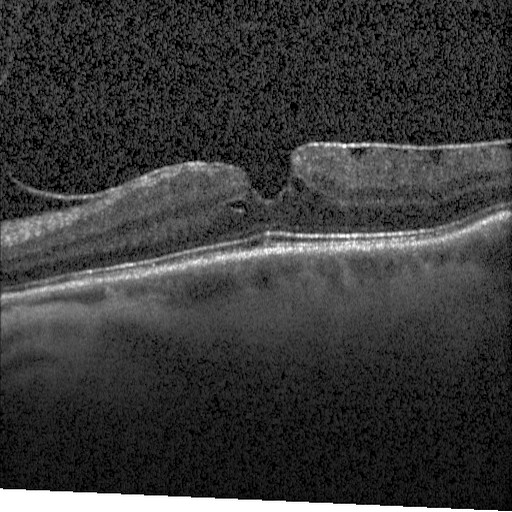 Centered on the fovea; optical coherence tomography B-scan; instrument: Heidelberg Spectralis. Impression: diabetic macular edema.